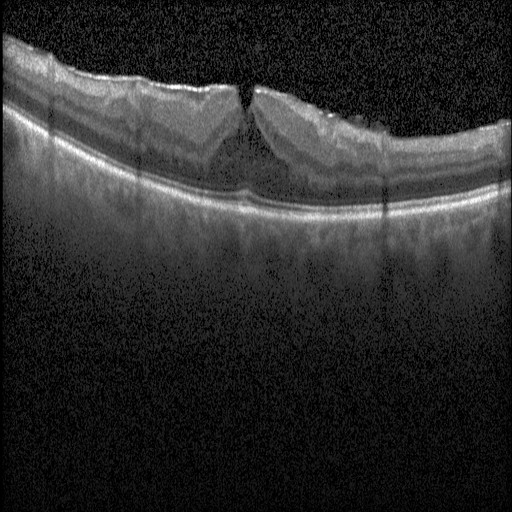

Spectral-domain optical coherence tomography, OCT B-scan
Impression: diabetic macular edema.